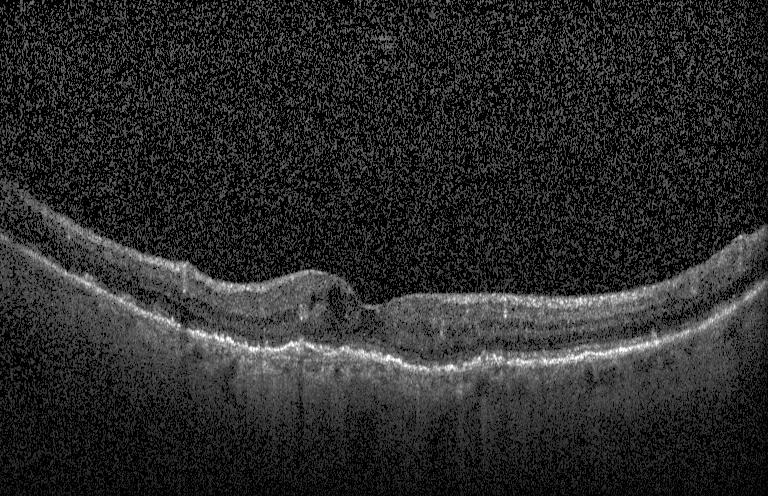

SD-OCT, Heidelberg Spectralis, OCT B-scan, through the macula
A choroidal neovascular membrane.